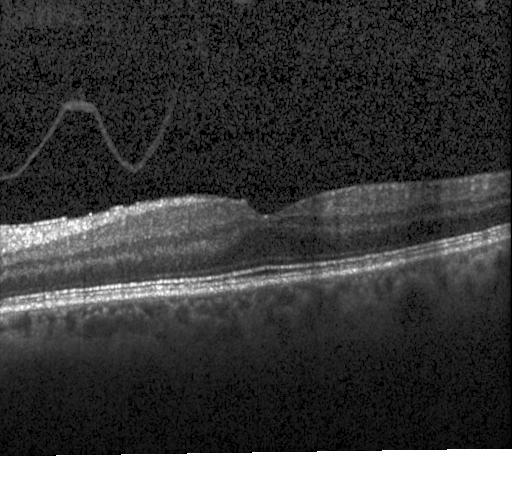
Optical coherence tomography B-scan
Dx: no choroidal neovascularization, diabetic macular edema, or drusen.